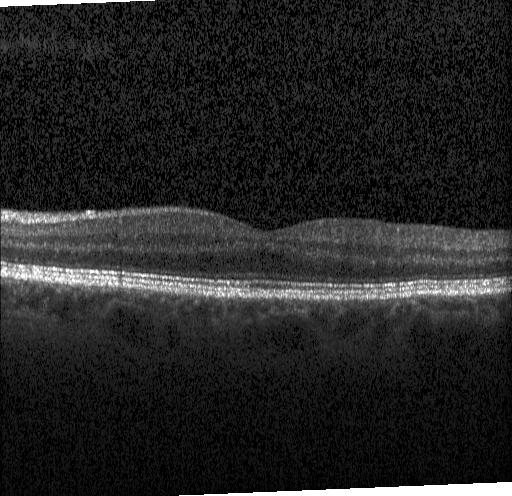
OCT scan showing no evidence of choroidal neovascularization, diabetic macular edema, or drusen.